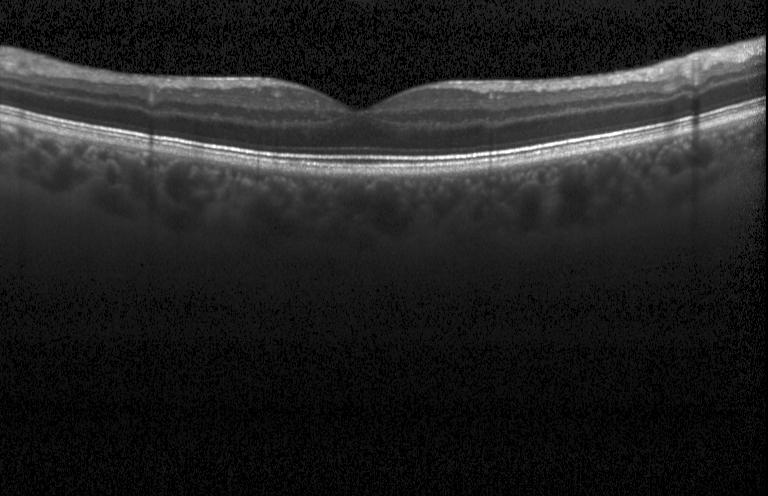 Retinal OCT cross-section showing neither CNV, DME, nor drusen.